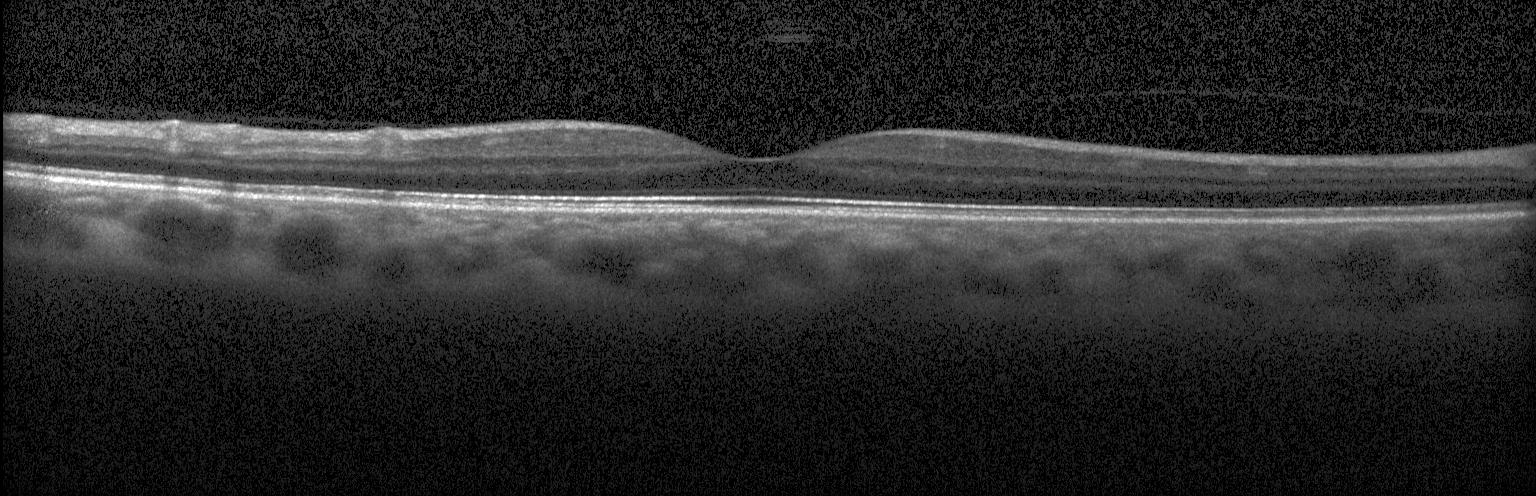

OCT line scan — Finding: no choroidal neovascularization, diabetic macular edema, or drusen.